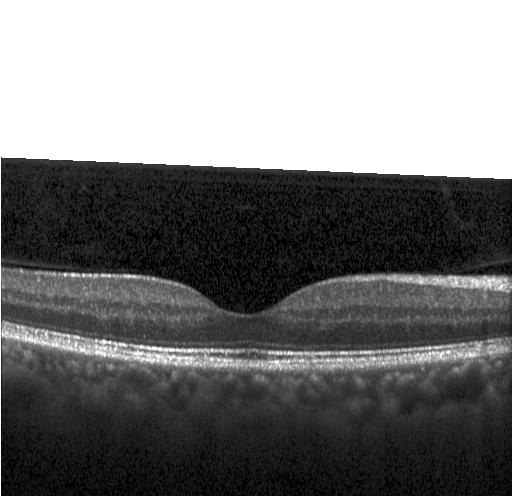
Impression: neither choroidal neovascularization, diabetic macular edema, nor drusen.